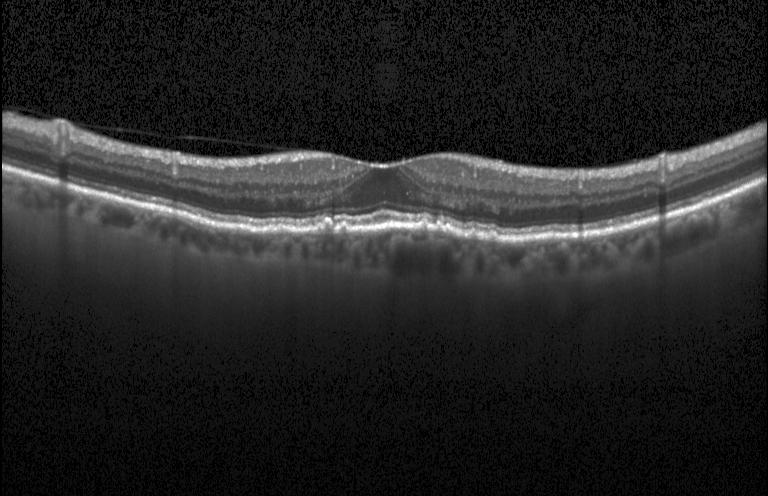
Optical coherence tomography B-scan. The scan shows multiple drusen.